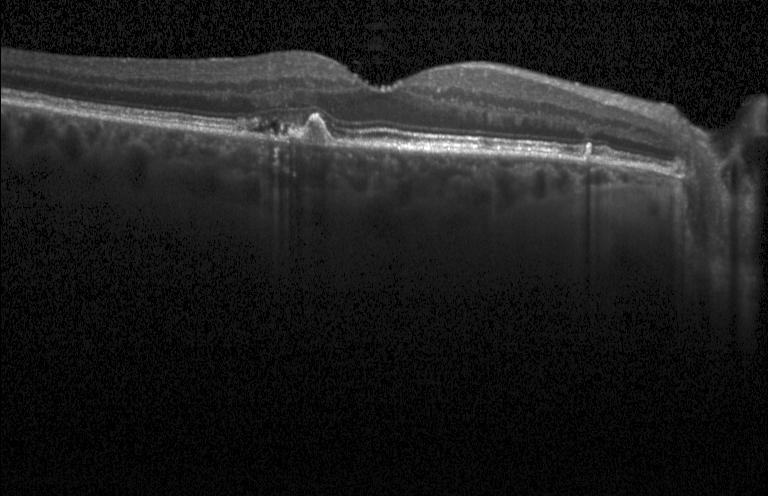

OCT line scan; acquired on a Heidelberg Spectralis. Impression: a choroidal neovascular membrane.